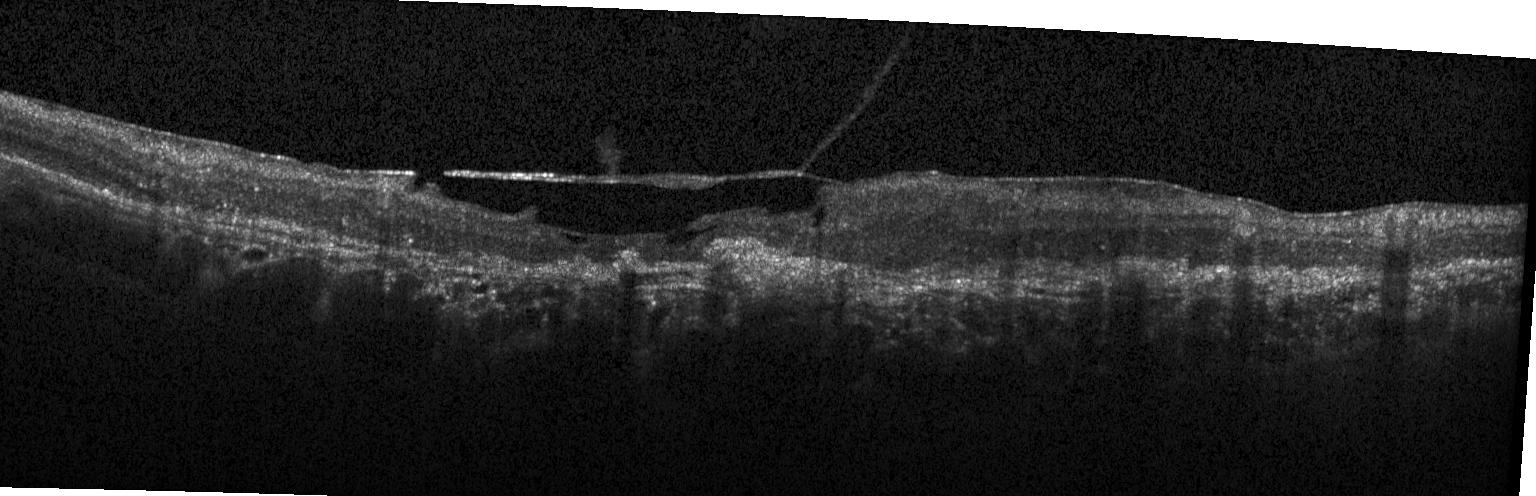 Optical coherence tomography scan.
Choroidal neovascularization.